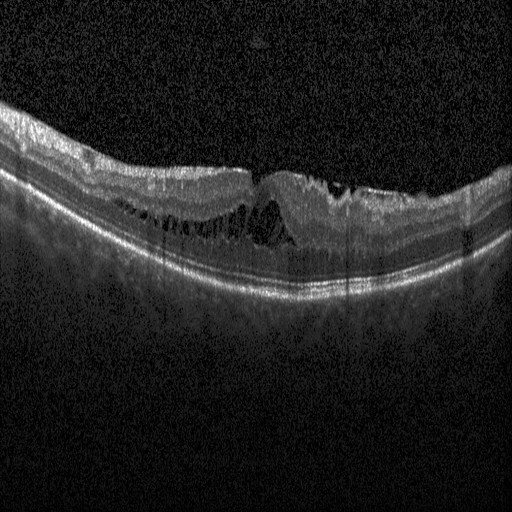 Retinal OCT B-scan — Finding: diabetic macular edema (DME).